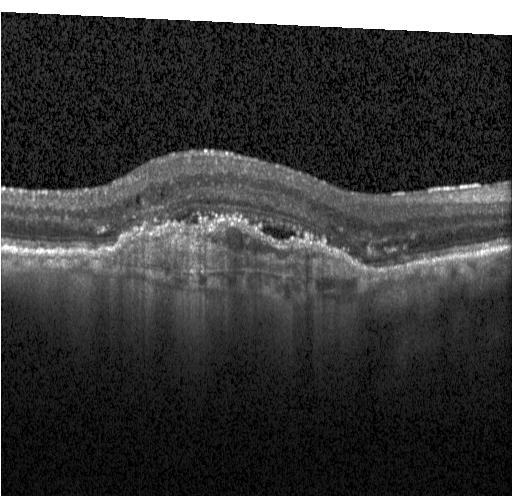 Spectral-domain OCT, OCT B-scan, Heidelberg Spectralis OCT system — Assessment: a choroidal neovascular membrane.